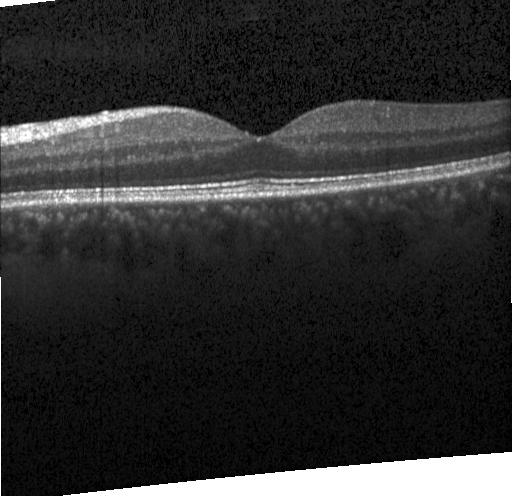
OCT B-scan showing no evidence of CNV, DME, or drusen.